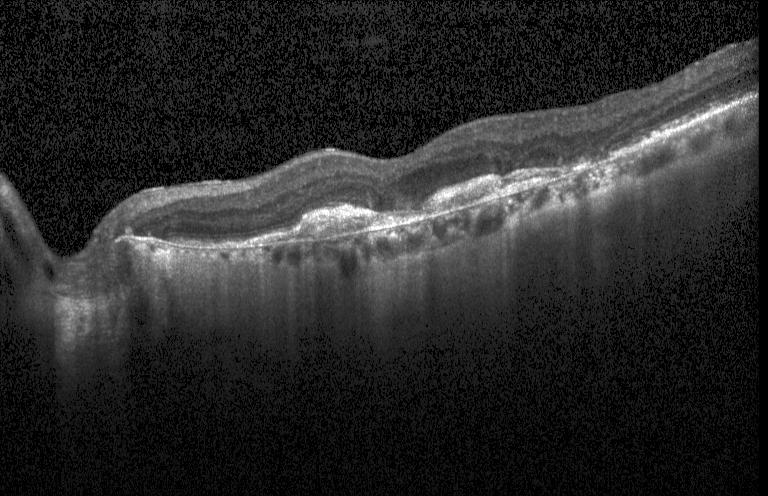 Retinal OCT B-scan.
Dx: CNV.